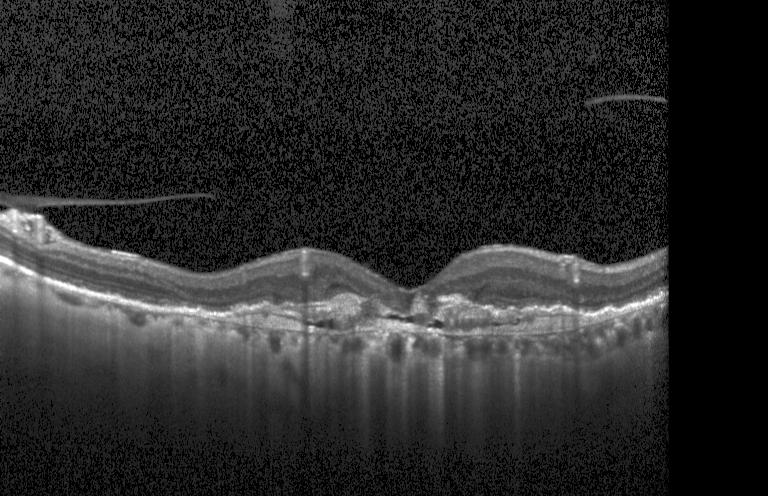

Optical coherence tomography scan
CNV.